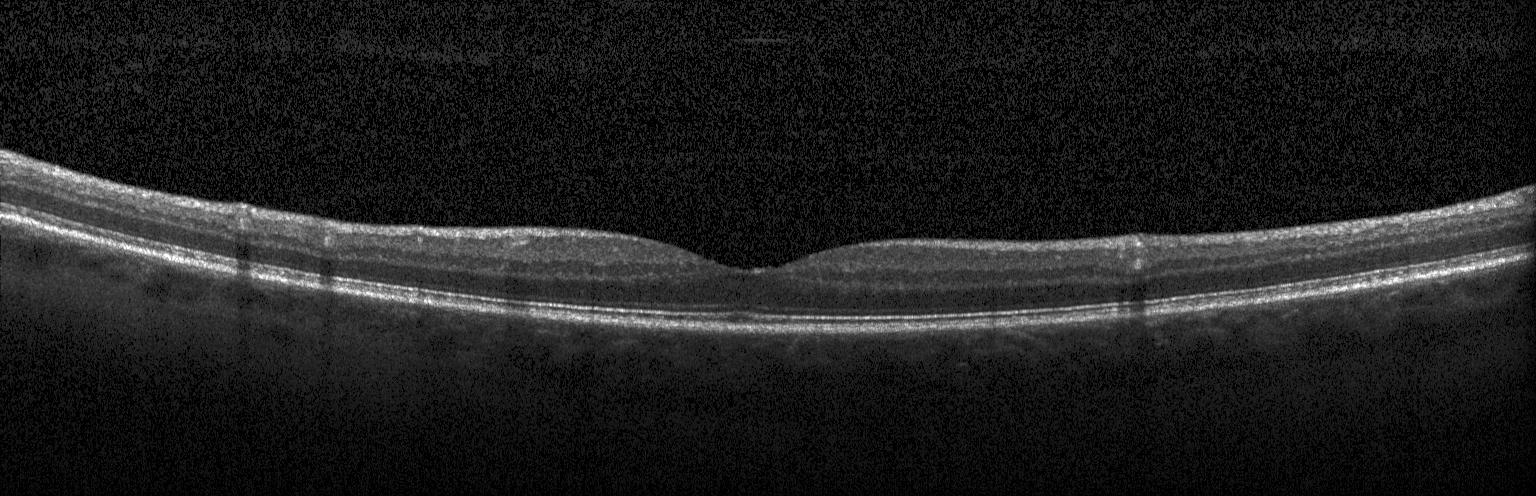

Retinal OCT B-scan. Macular scan. Acquired on a Heidelberg Spectralis. Spectral-domain OCT — Macular OCT: neither choroidal neovascularization, diabetic macular edema, nor drusen.